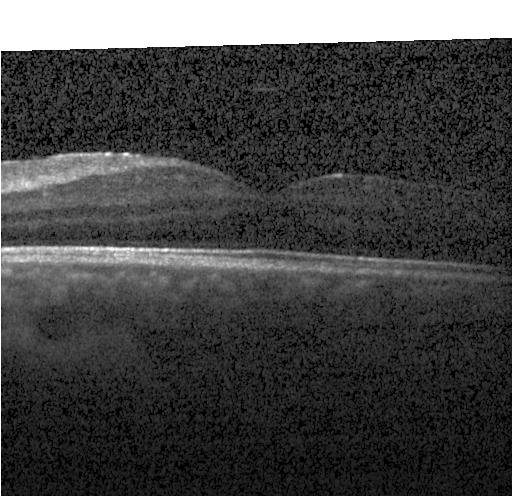
Spectral-domain OCT B-scan: no choroidal neovascularization, no diabetic macular edema, and no drusen.